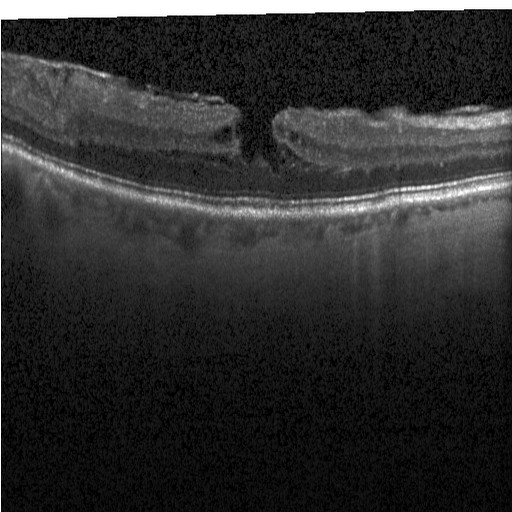 Optical coherence tomography scan, Heidelberg Spectralis, macular scan — Diagnosis: DME.